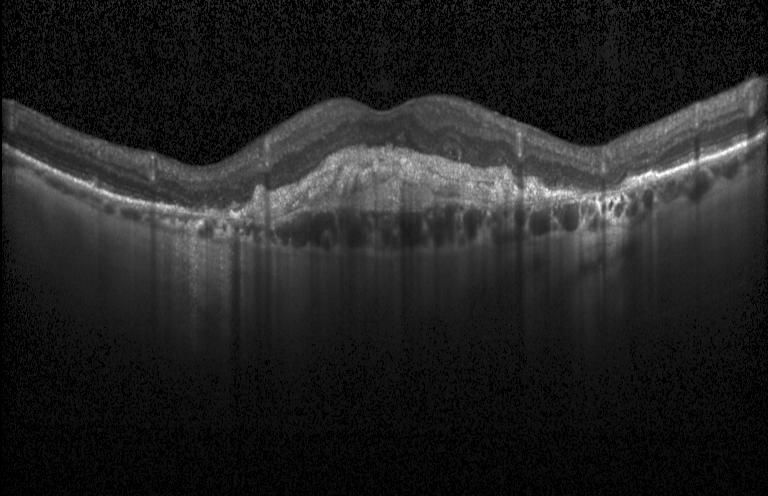 Finding: a choroidal neovascular membrane.